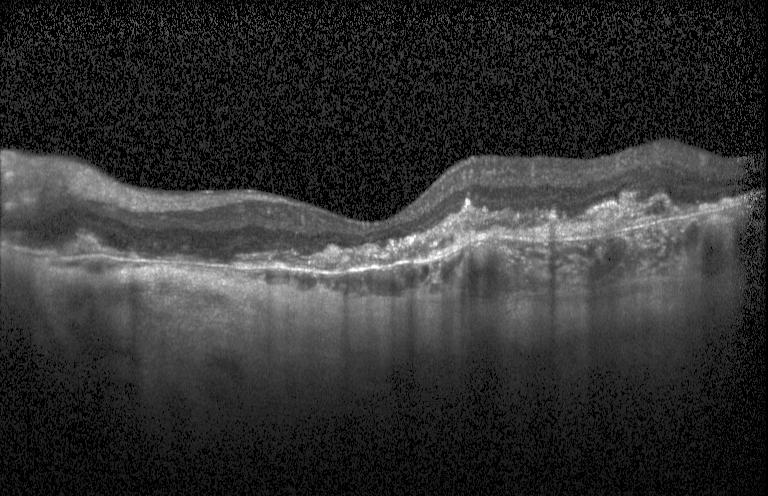
Acquired on a Heidelberg Spectralis · OCT B-scan. A choroidal neovascular membrane.